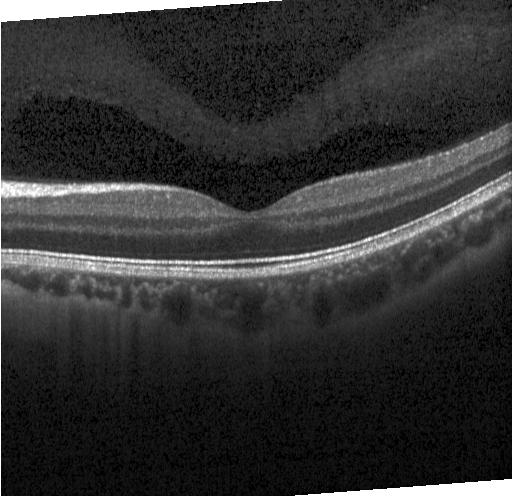 Heidelberg Spectralis OCT system; retinal OCT cross-section; spectral-domain optical coherence tomography; macular scan. OCT finding: no choroidal neovascularization, no diabetic macular edema, and no drusen.